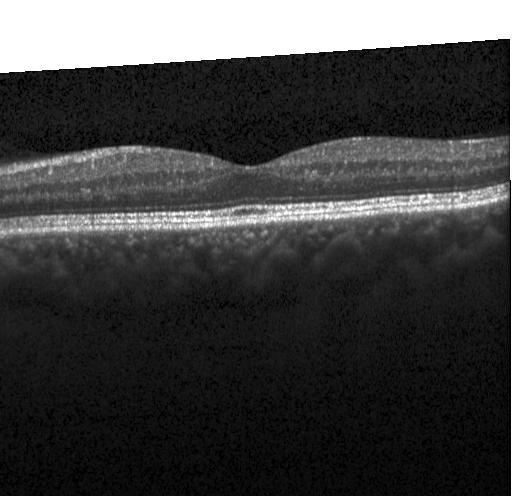 OCT B-scan; Heidelberg Spectralis. Assessment: neither CNV, DME, nor drusen.